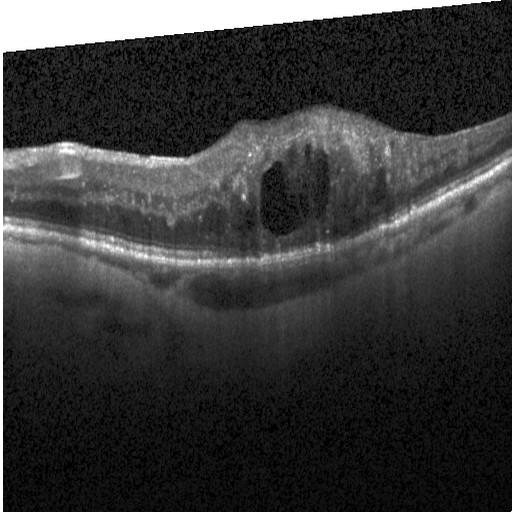

Spectral-domain OCT B-scan: diabetic macular edema (DME).